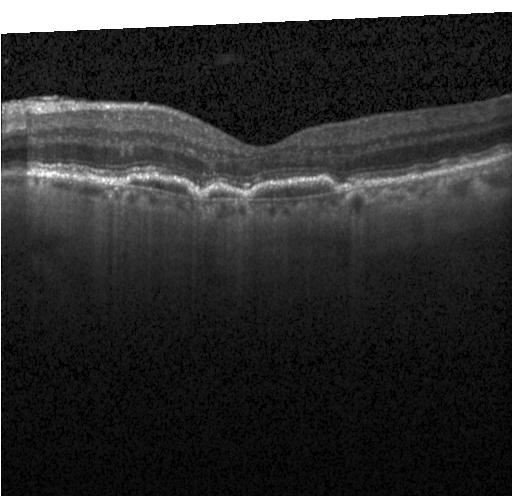 OCT line scan; instrument: Heidelberg Spectralis; spectral-domain optical coherence tomography
The scan shows a choroidal neovascular membrane.